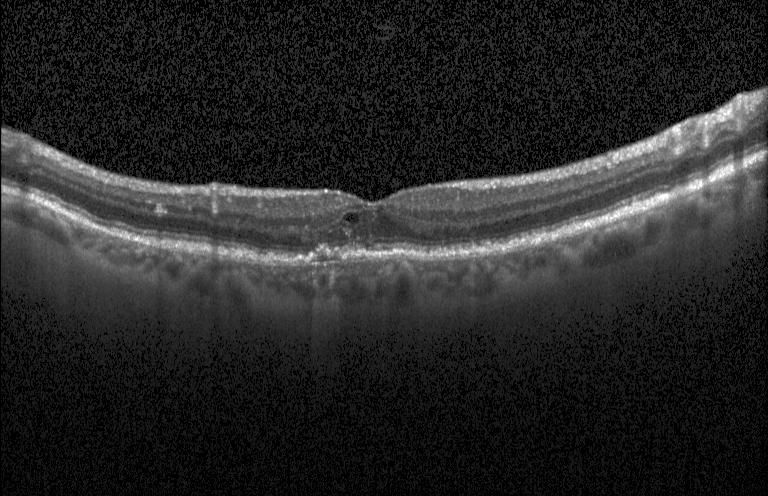
Finding: a choroidal neovascular membrane.